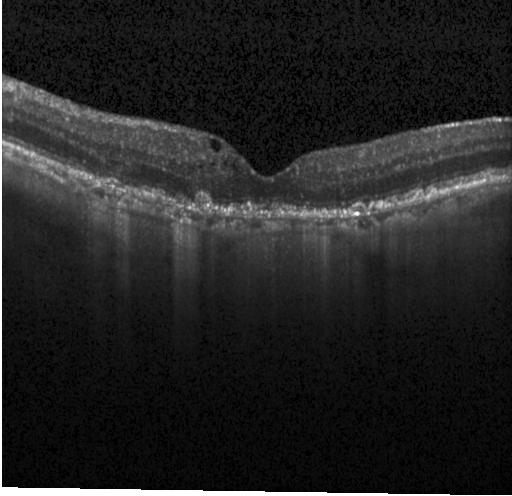
Macular OCT: a choroidal neovascular membrane.